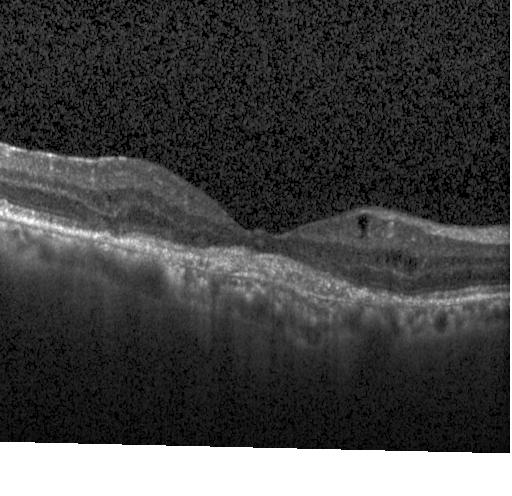 OCT line scan. Fovea-centered. Spectral-domain optical coherence tomography
Impression: a choroidal neovascular membrane.